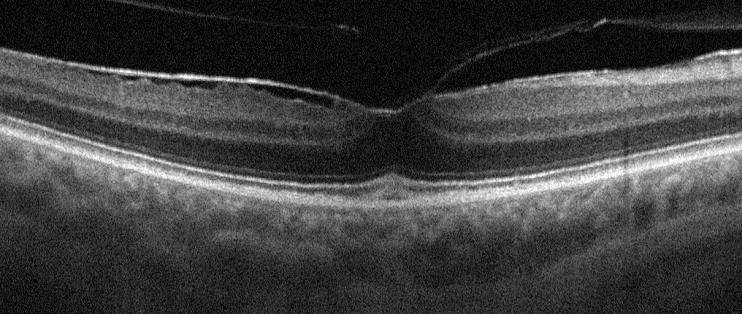
Optical coherence tomography scan — This B-scan demonstrates epiretinal membrane (ERM).